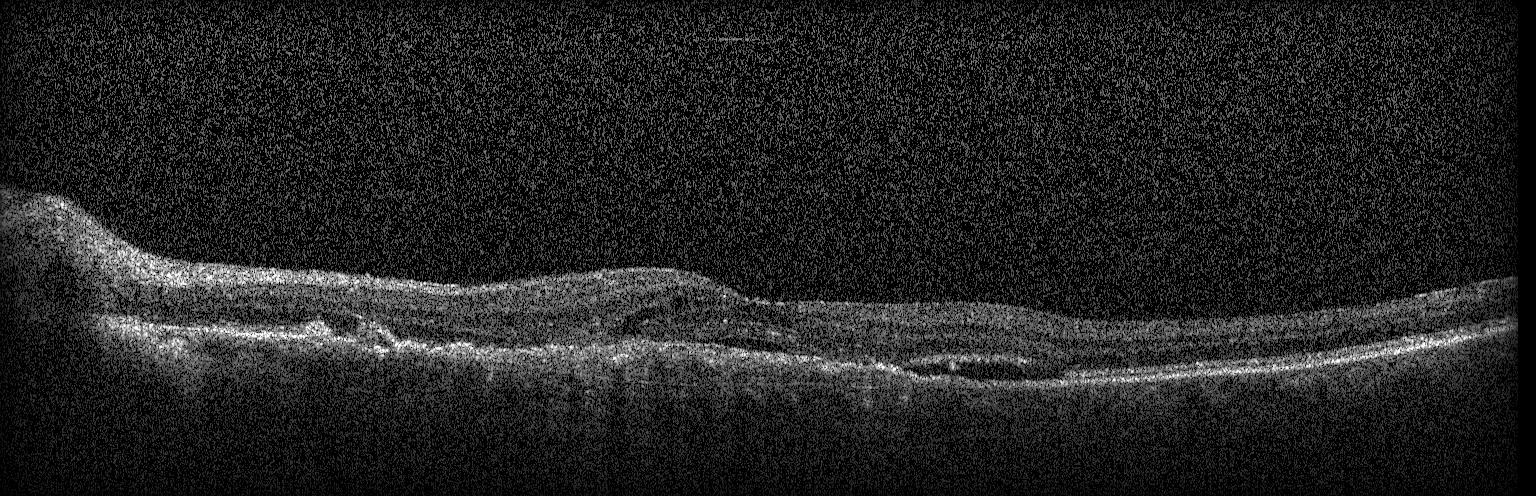
Retinal OCT cross-section. Diagnosis: choroidal neovascularization.